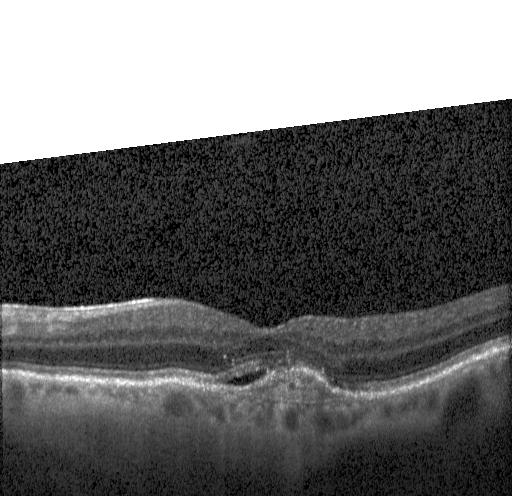 Finding: a choroidal neovascular membrane.